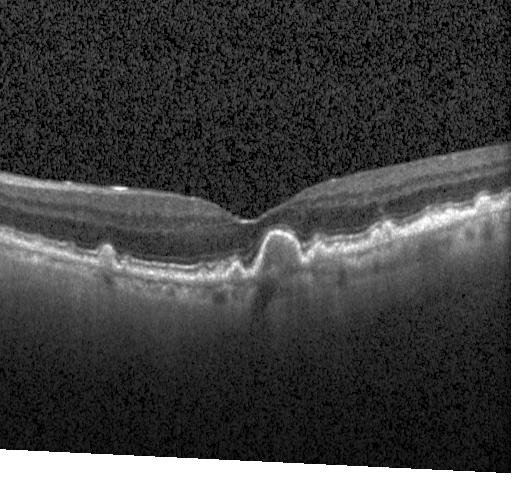

Optical coherence tomography B-scan. Finding: multiple drusen.